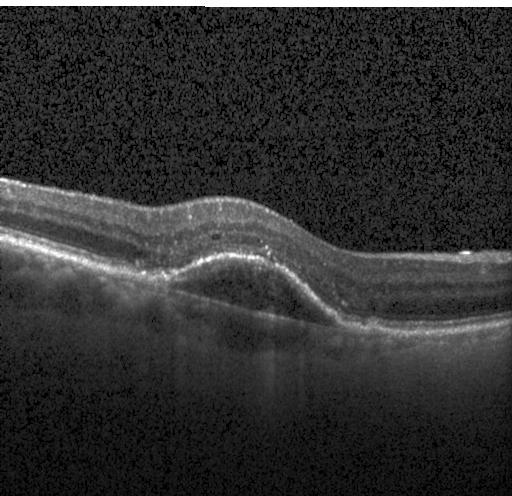 Optical coherence tomography B-scan · macular scan.
Dx: a choroidal neovascular membrane.